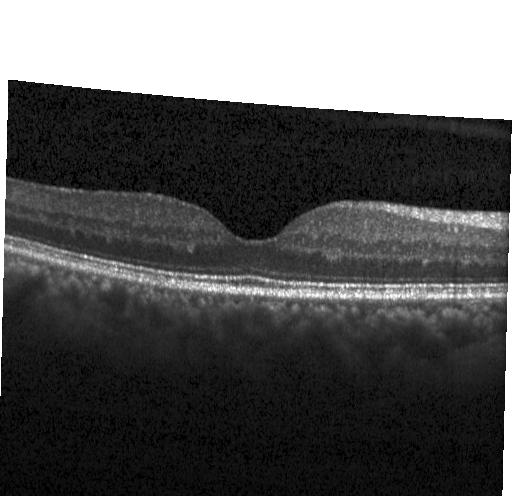
Spectral-domain OCT B-scan: no evidence of choroidal neovascularization, diabetic macular edema, or drusen.